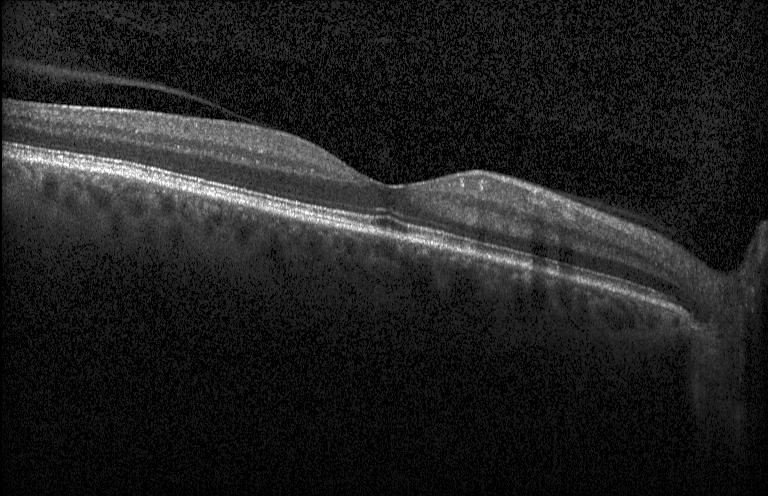 OCT B-scan · acquired on a Heidelberg Spectralis · centered on the fovea · SD-OCT.
Diagnosis: no CNV, no DME, and no drusen.